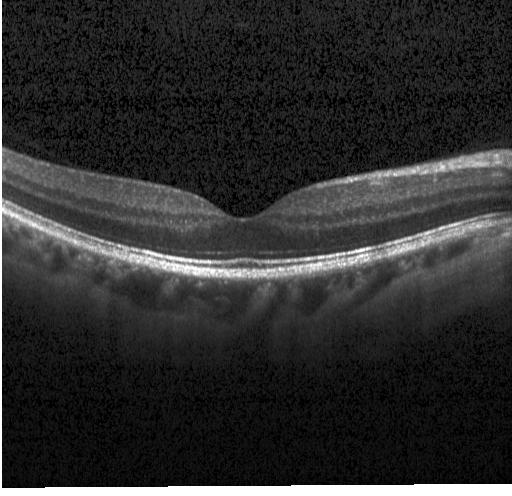 Optical coherence tomography B-scan · centered on the fovea · SD-OCT · Heidelberg Spectralis — Assessment: no choroidal neovascularization, diabetic macular edema, or drusen.